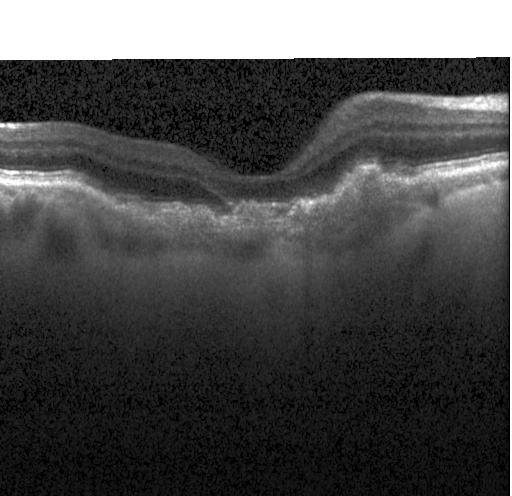 Finding: a choroidal neovascular membrane.